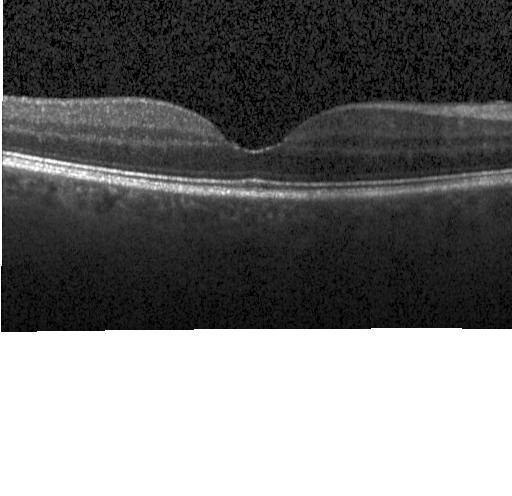
Spectral-domain OCT, fovea-centered, retinal OCT B-scan
Finding: no choroidal neovascularization, no diabetic macular edema, and no drusen.